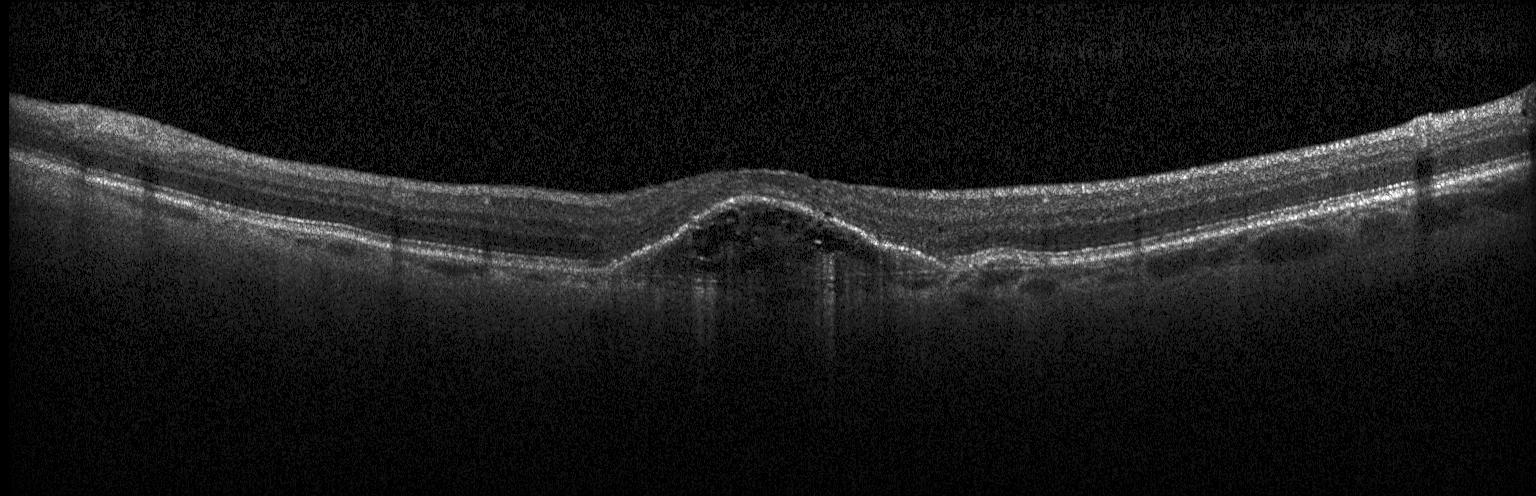
Retinal OCT B-scan · Heidelberg Spectralis OCT system · spectral-domain OCT
This B-scan demonstrates CNV.